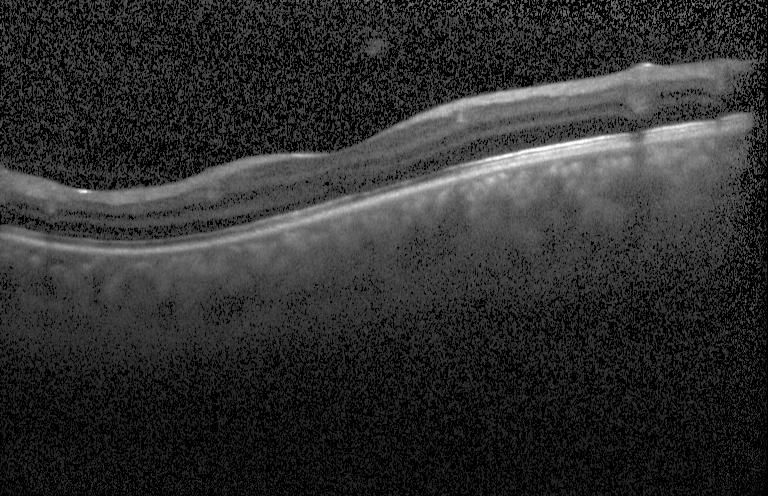
OCT B-scan showing neither choroidal neovascularization, diabetic macular edema, nor drusen.